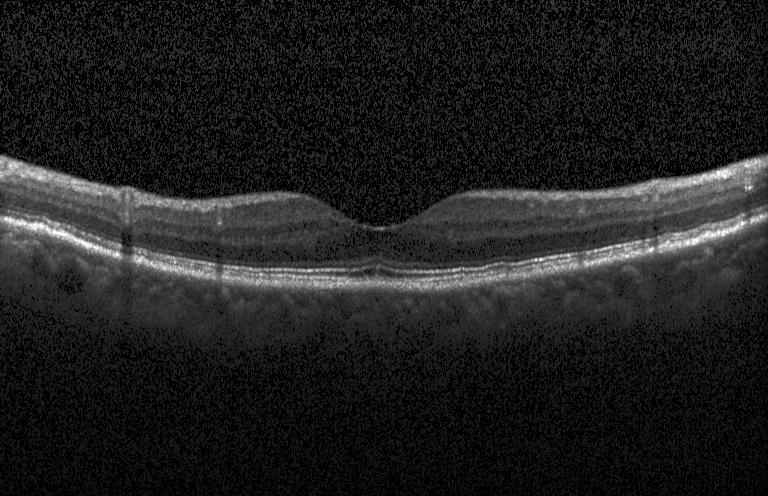
Retinal OCT B-scan · SD-OCT — Diagnosis: no choroidal neovascularization, no diabetic macular edema, and no drusen.